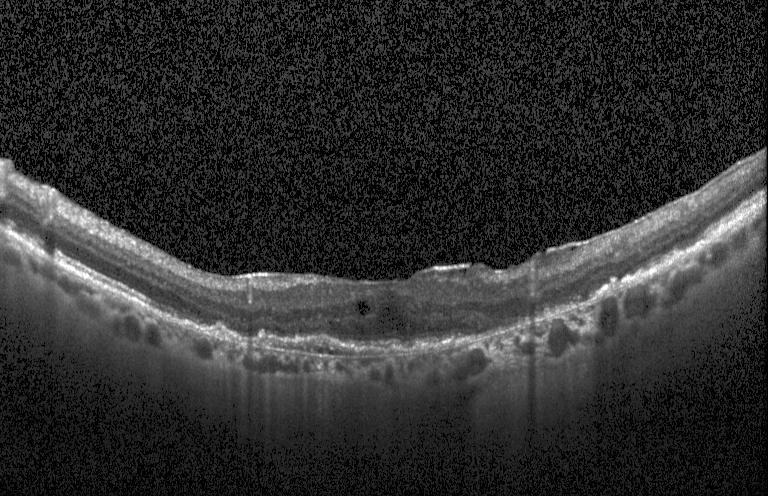

OCT line scan — This B-scan demonstrates a choroidal neovascular membrane.